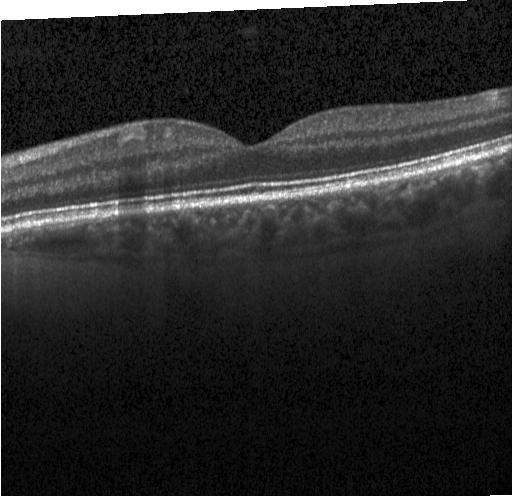
OCT finding: no choroidal neovascularization, diabetic macular edema, or drusen.